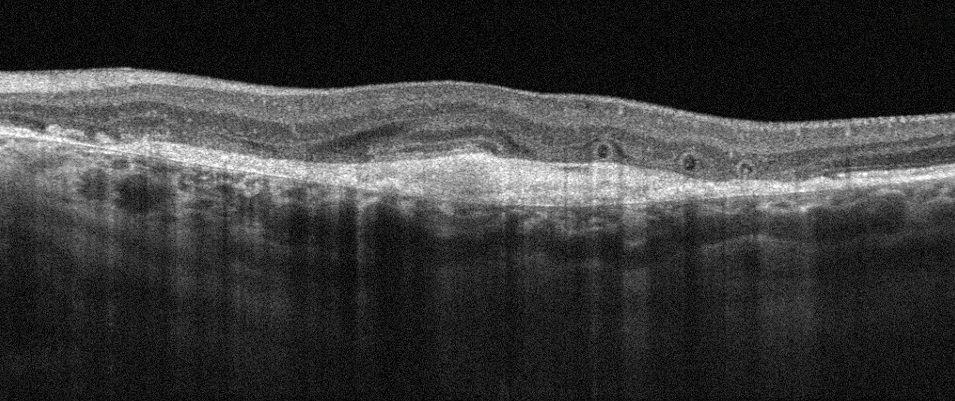
OCT B-scan, macular scan, acquired on an Optovue Avanti RTVue XR.
The scan shows AMD.